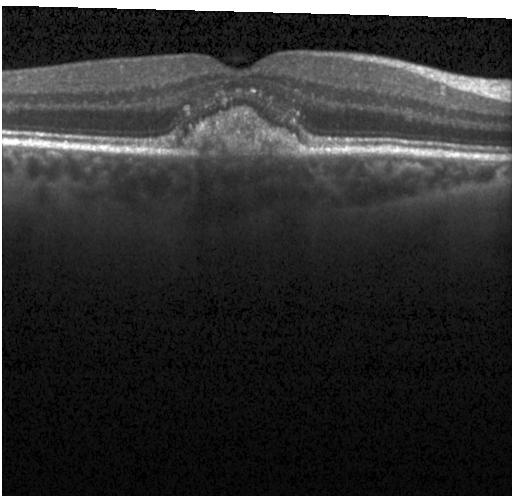
Optical coherence tomography B-scan · macular scan.
The scan shows a choroidal neovascular membrane.